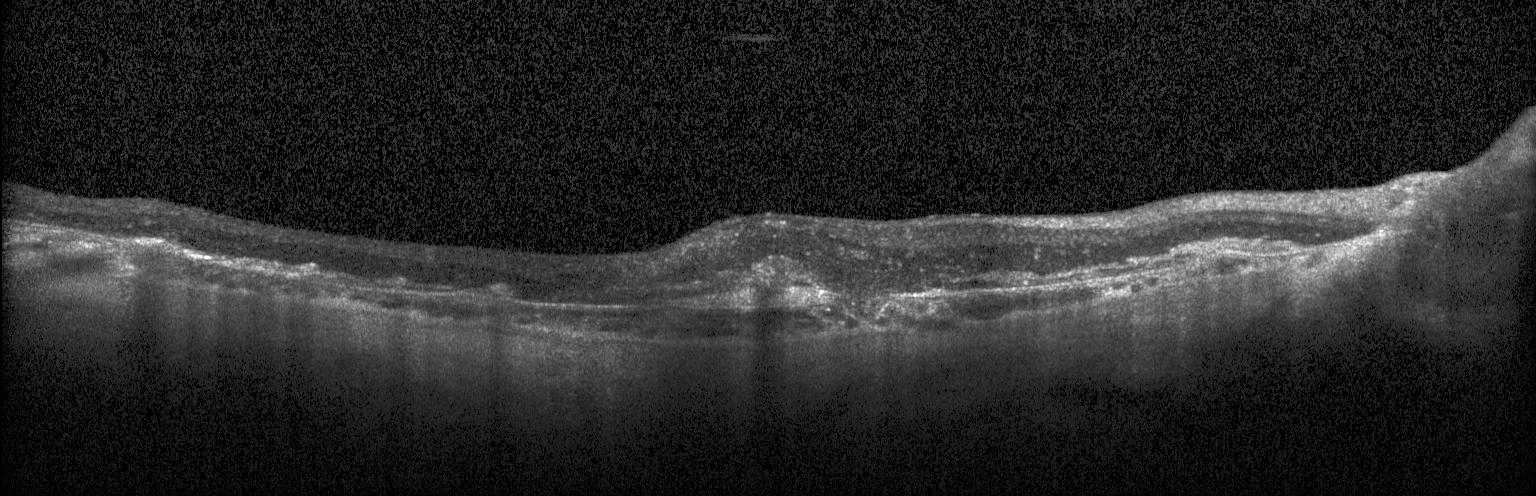

OCT B-scan showing a choroidal neovascular membrane.